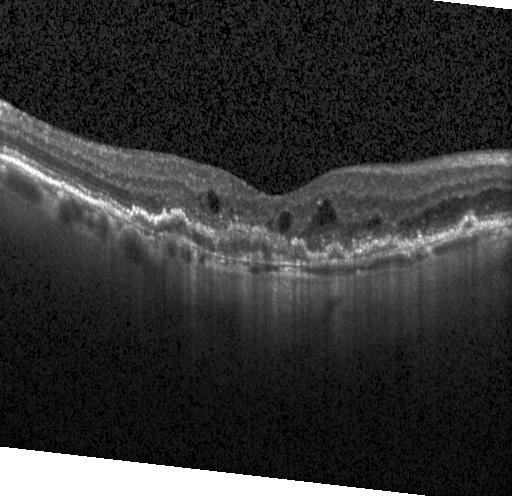 Heidelberg Spectralis · horizontal scan through the fovea · spectral-domain optical coherence tomography · OCT line scan
This B-scan demonstrates a choroidal neovascular membrane.